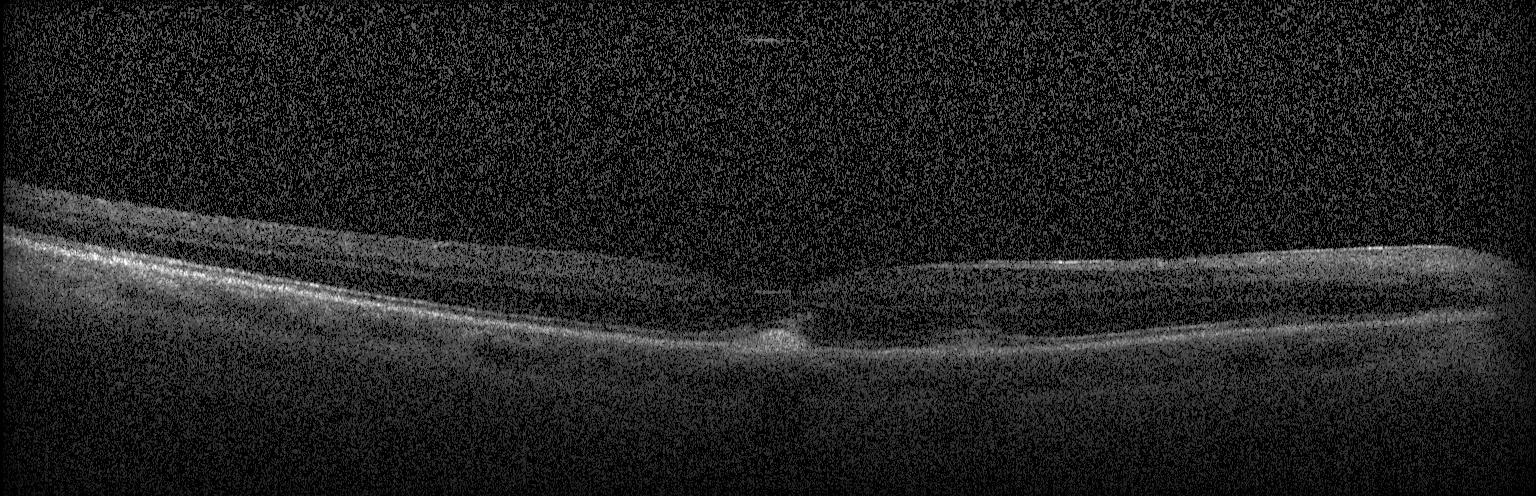
Macular OCT: a choroidal neovascular membrane.